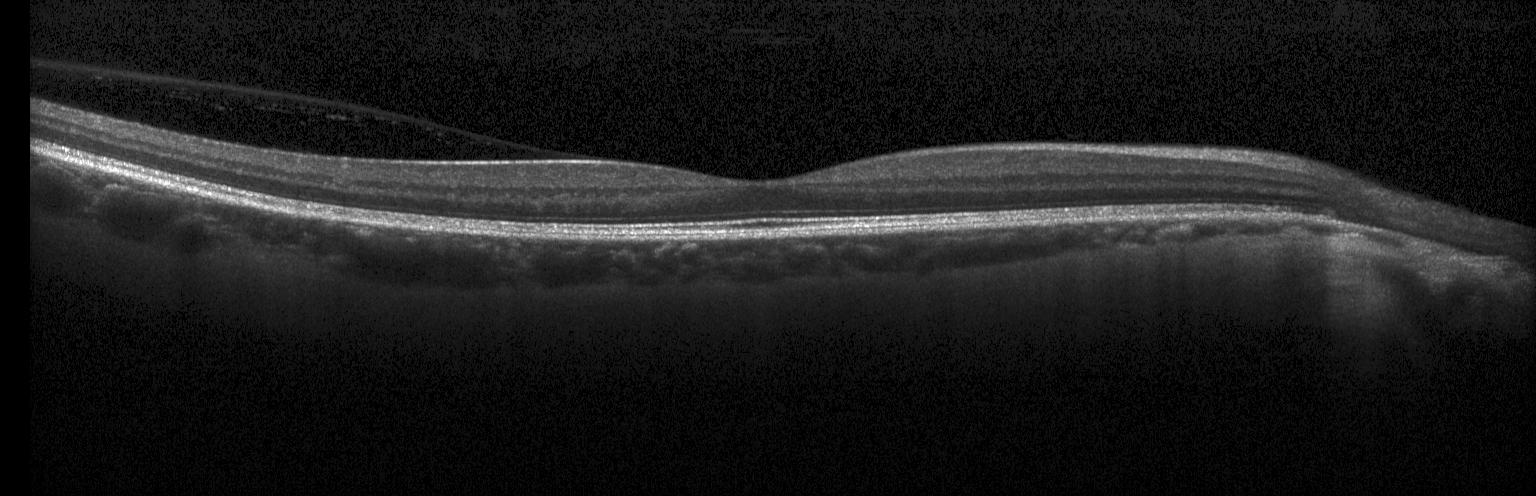 Finding: no choroidal neovascularization, diabetic macular edema, or drusen.